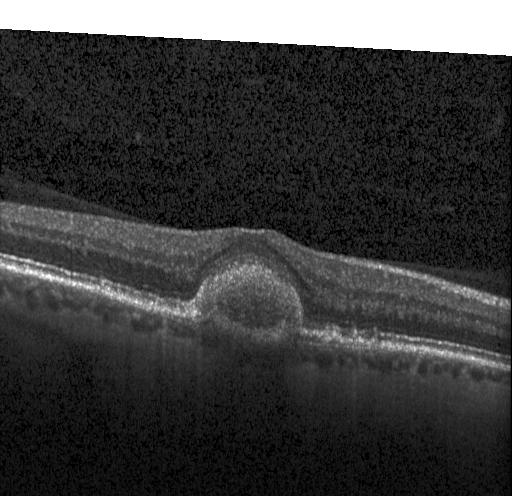 Dx: a choroidal neovascular membrane.